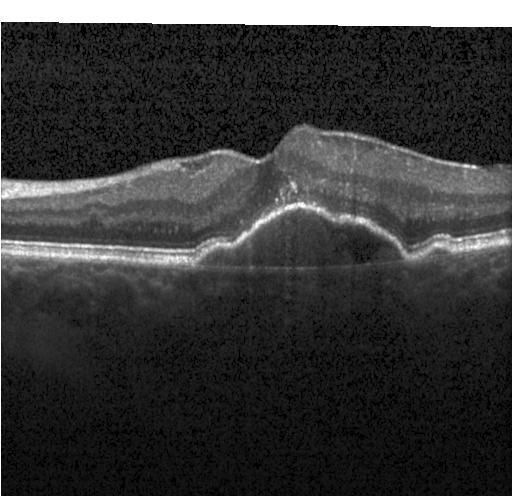 Optical coherence tomography scan; acquired on a Heidelberg Spectralis; horizontal scan through the fovea
Impression: choroidal neovascularization (CNV).